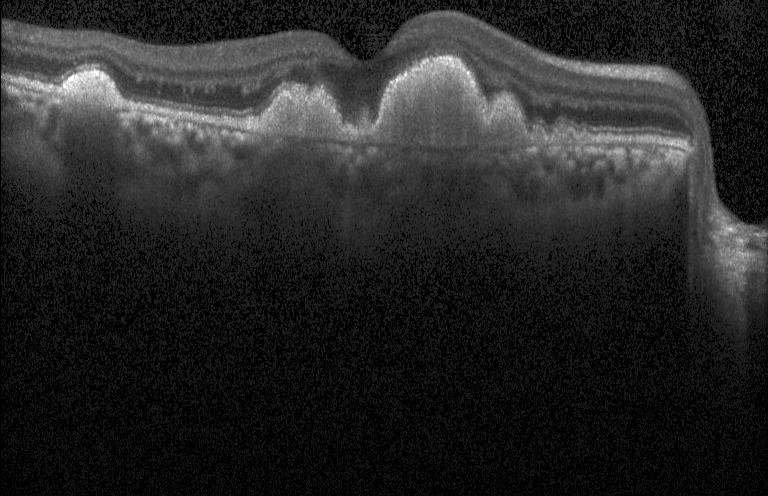 OCT B-scan — Impression: drusen.